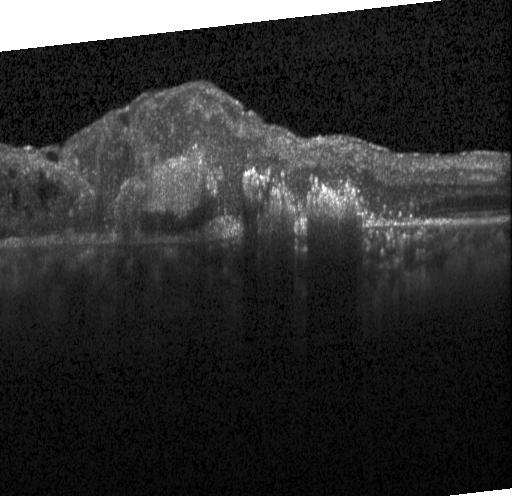
Instrument: Heidelberg Spectralis, optical coherence tomography B-scan — Choroidal neovascularization.